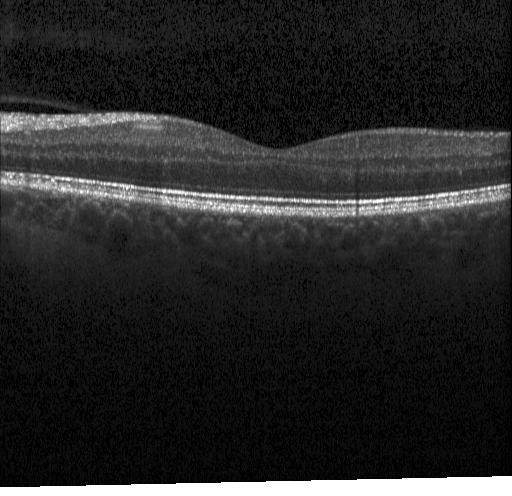 Through the macula · spectral-domain optical coherence tomography · OCT B-scan. Finding: neither CNV, DME, nor drusen.